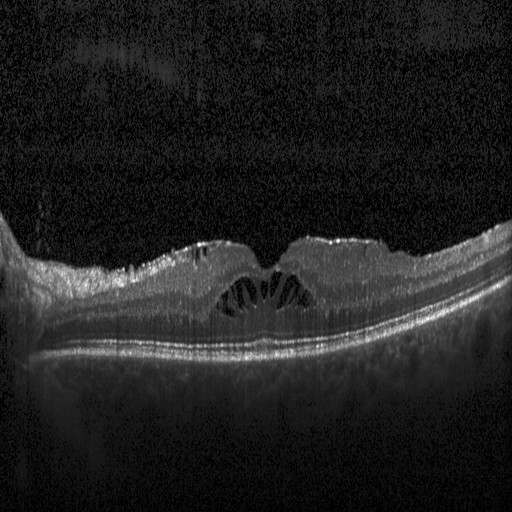
Retinal OCT cross-section showing DME.